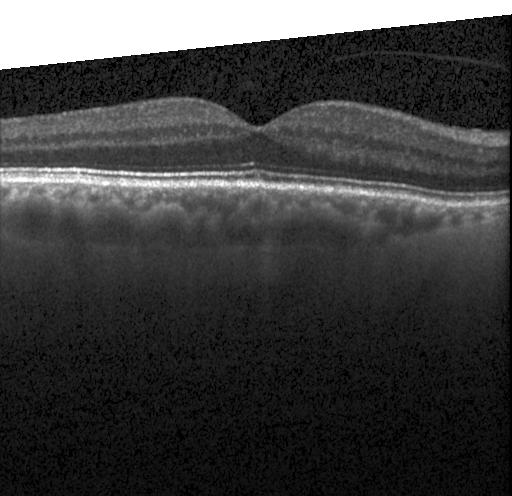 Heidelberg Spectralis OCT system · optical coherence tomography scan.
Impression: neither choroidal neovascularization, diabetic macular edema, nor drusen.